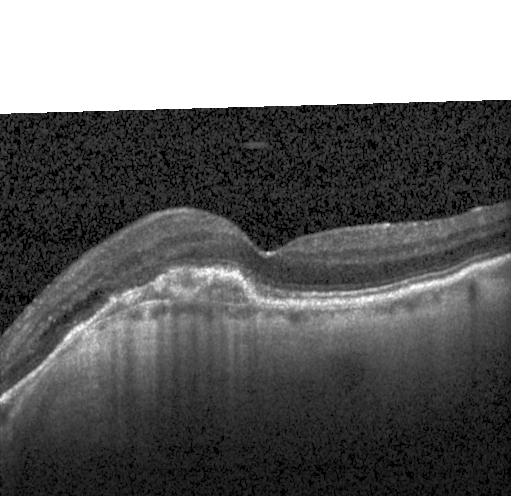

OCT line scan — Macular OCT: a choroidal neovascular membrane.